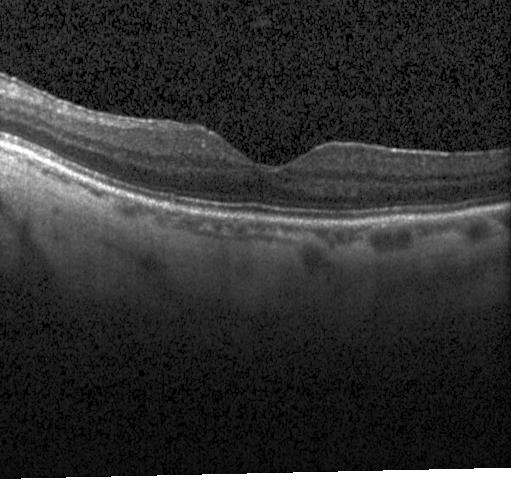

OCT B-scan; fovea-centered.
Finding: no CNV, no DME, and no drusen.